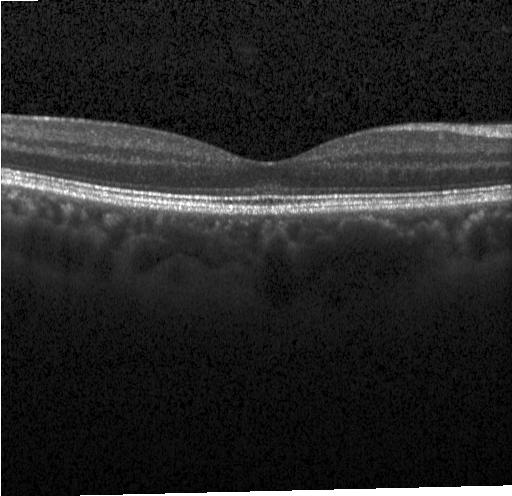
Spectral-domain OCT. Through the macula. OCT line scan. Dx: no evidence of CNV, DME, or drusen.